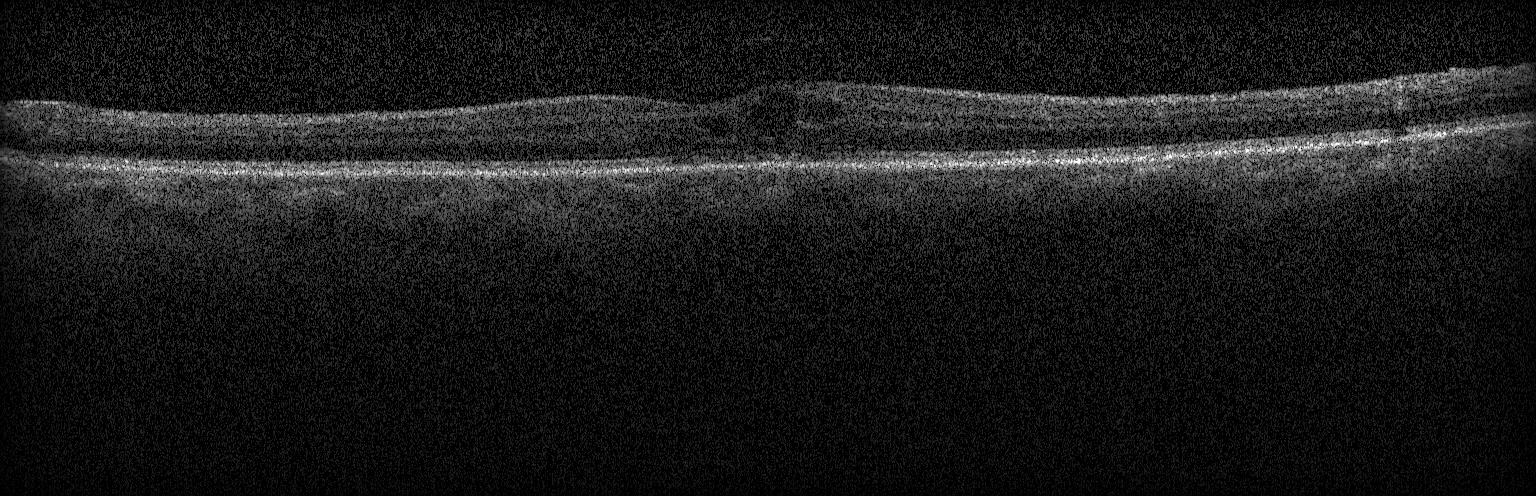
Horizontal scan through the fovea · OCT line scan. Diabetic macular edema (DME).